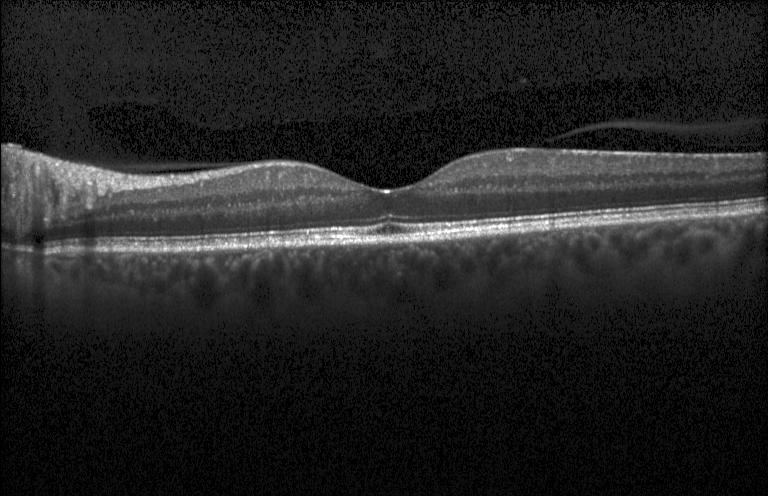
SD-OCT. Macular scan. Heidelberg Spectralis. Retinal OCT cross-section.
Finding: no evidence of CNV, DME, or drusen.